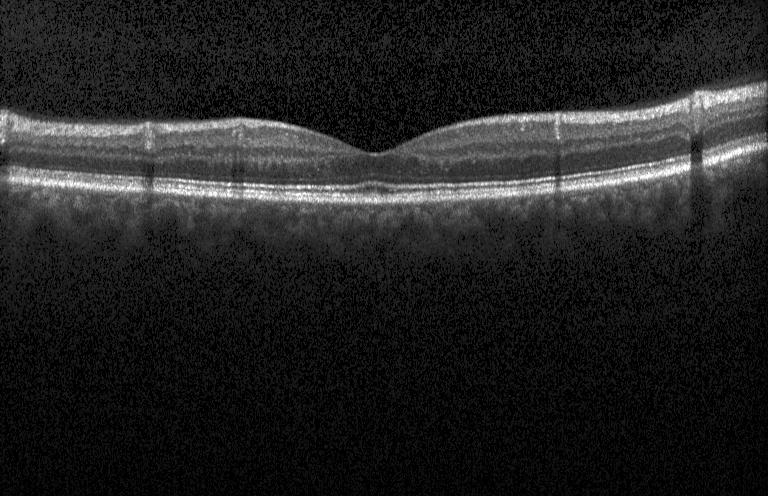

Instrument: Heidelberg Spectralis. Optical coherence tomography B-scan. Dx: no evidence of choroidal neovascularization, diabetic macular edema, or drusen.